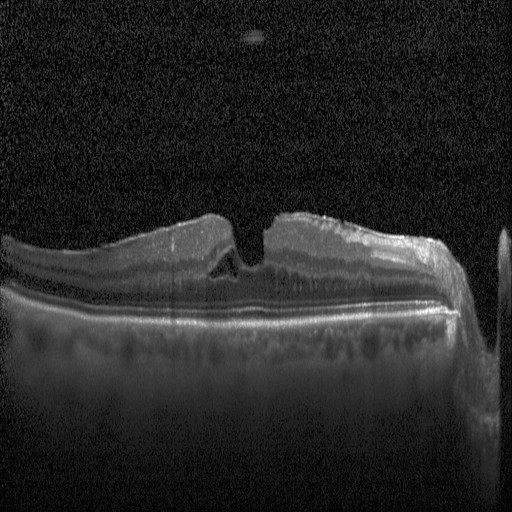
Spectral-domain OCT · optical coherence tomography scan · horizontal scan through the fovea · Heidelberg Spectralis OCT system — This B-scan demonstrates diabetic macular edema.